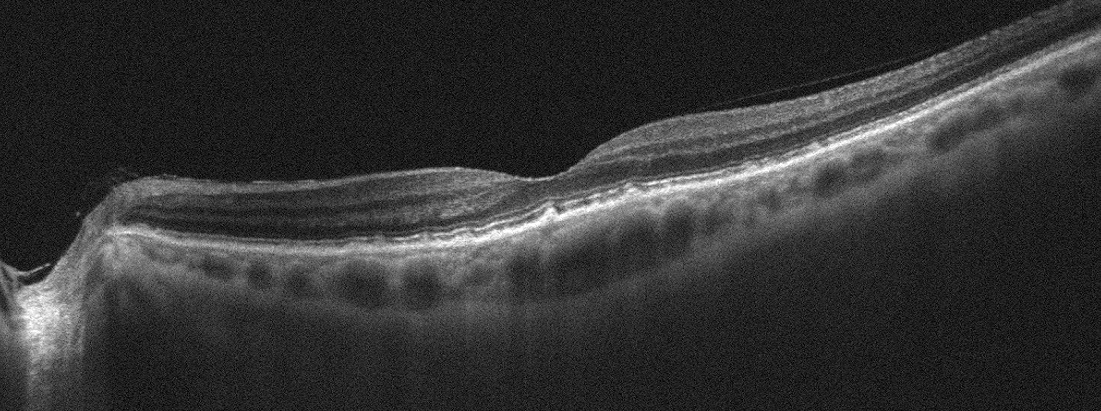
Finding: age-related macular degeneration (AMD).